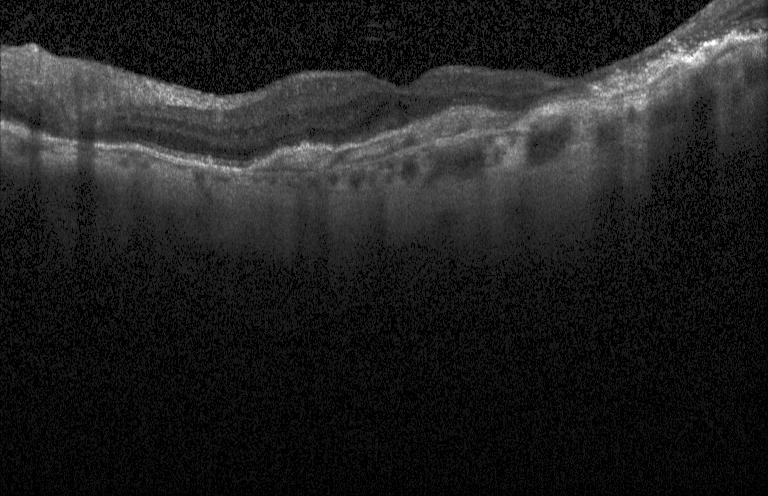

Through the macula · retinal OCT B-scan
Macular OCT: a choroidal neovascular membrane.